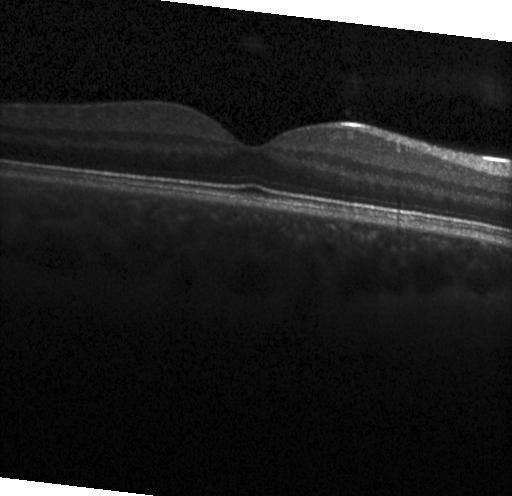 OCT B-scan showing neither choroidal neovascularization, diabetic macular edema, nor drusen.